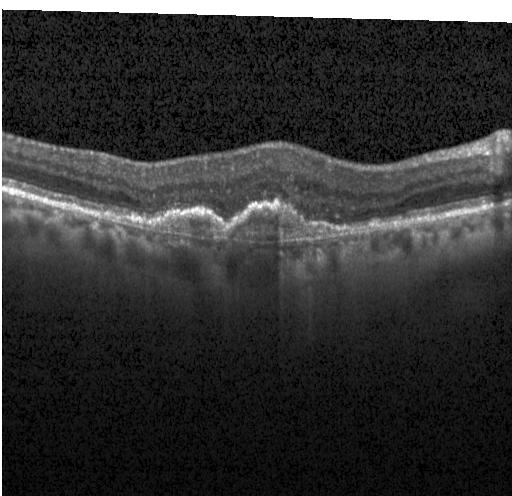
SD-OCT. Through the macula. OCT B-scan. Heidelberg Spectralis. OCT finding: a choroidal neovascular membrane.